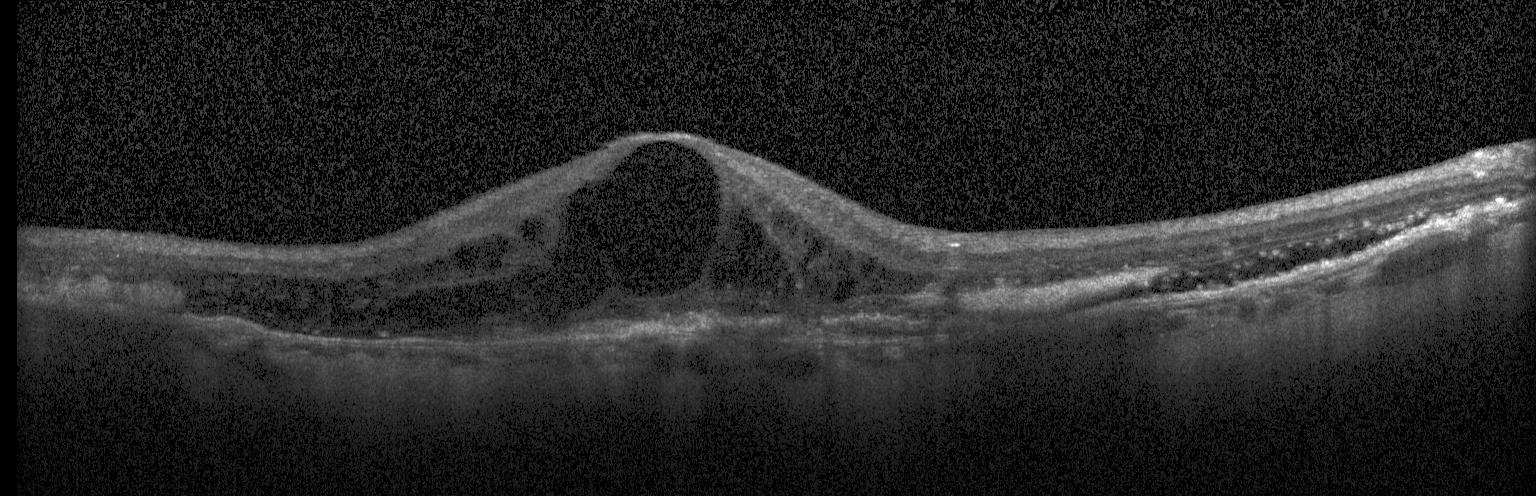

Fovea-centered, Heidelberg Spectralis, SD-OCT, retinal OCT B-scan.
Diagnosis: choroidal neovascularization.